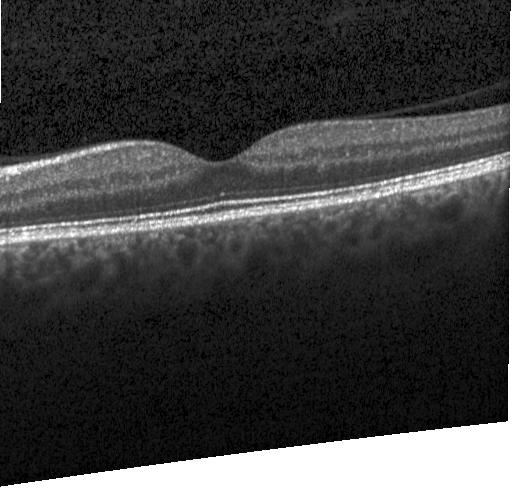
Diagnosis: no evidence of CNV, DME, or drusen.